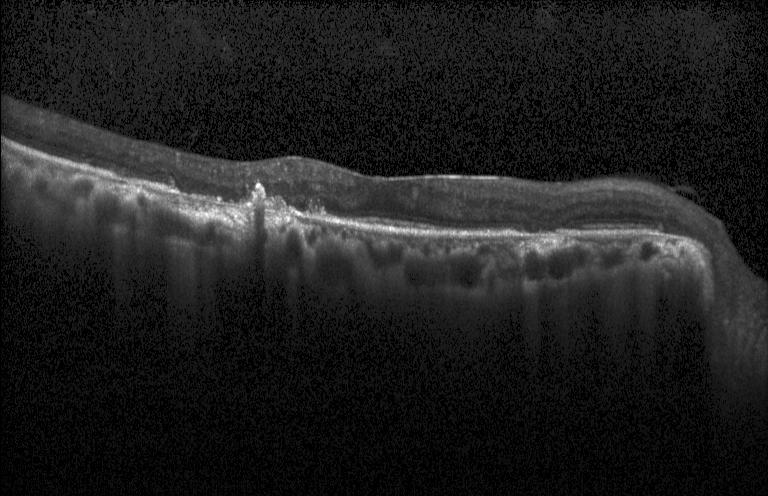
Spectral-domain OCT · centered on the fovea · retinal OCT cross-section · Heidelberg Spectralis OCT system — Diagnosis: a choroidal neovascular membrane.